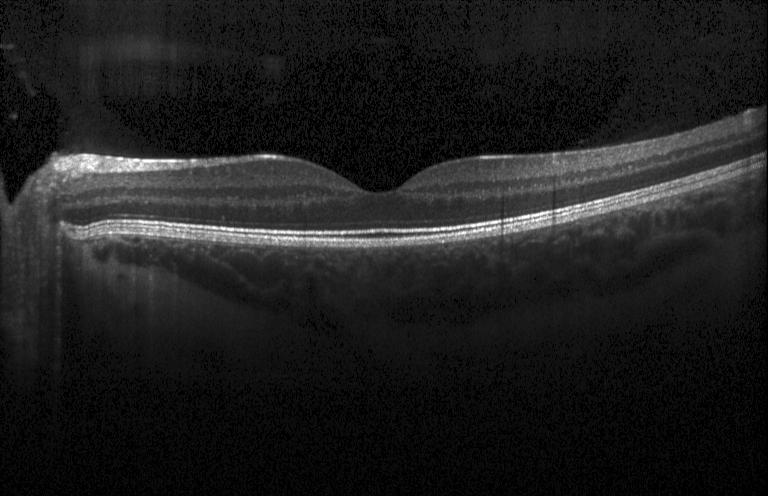 Spectral-domain optical coherence tomography. Instrument: Heidelberg Spectralis. Centered on the fovea. OCT line scan — Impression: no evidence of choroidal neovascularization, diabetic macular edema, or drusen.